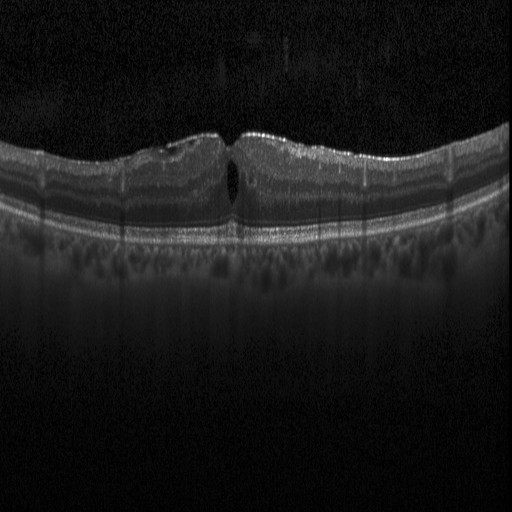
OCT B-scan.
Diabetic macular edema (DME).